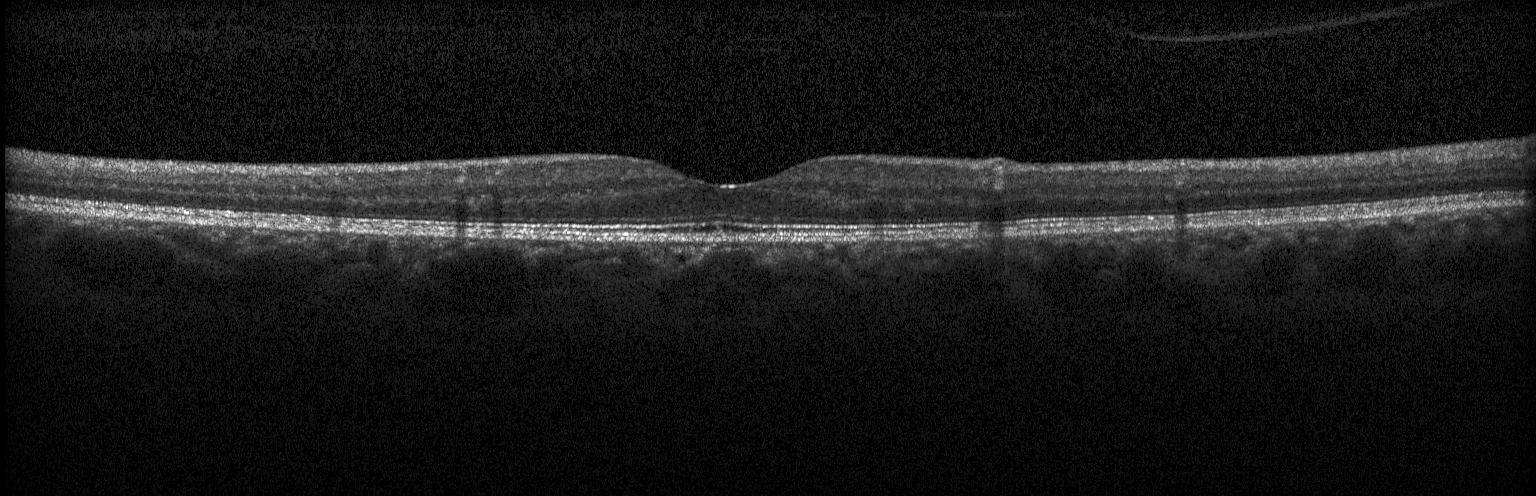
Horizontal scan through the fovea · retinal OCT cross-section · SD-OCT · acquired on a Heidelberg Spectralis — Diagnosis: neither CNV, DME, nor drusen.